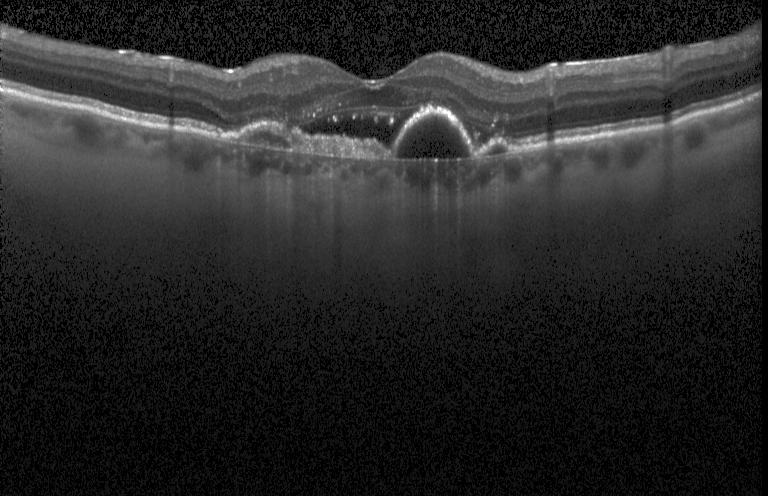

Spectral-domain OCT, retinal OCT B-scan, centered on the fovea, acquired on a Heidelberg Spectralis.
Dx: choroidal neovascularization (CNV).